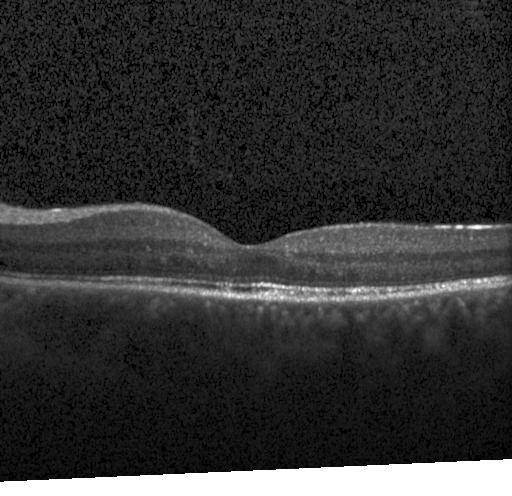

OCT line scan, spectral-domain OCT, horizontal scan through the fovea.
OCT finding: no evidence of choroidal neovascularization, diabetic macular edema, or drusen.